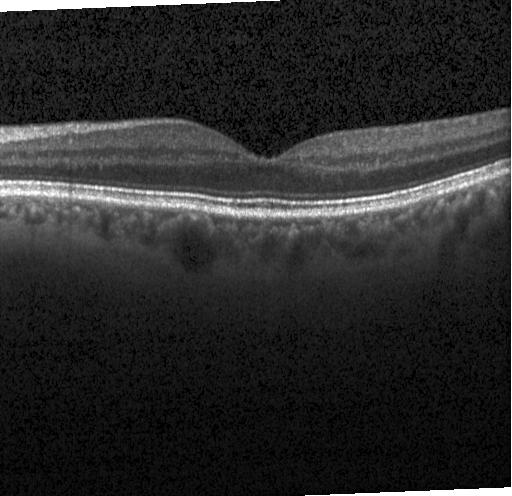
Impression: no evidence of CNV, DME, or drusen.